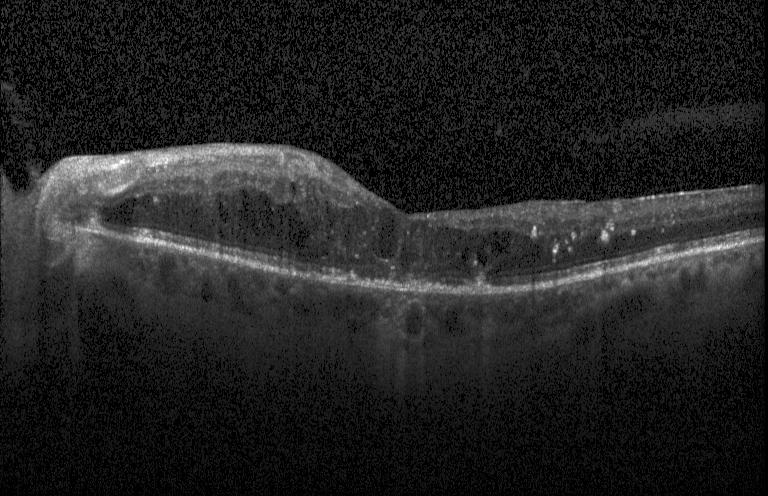 Horizontal scan through the fovea; optical coherence tomography scan. Impression: DME.